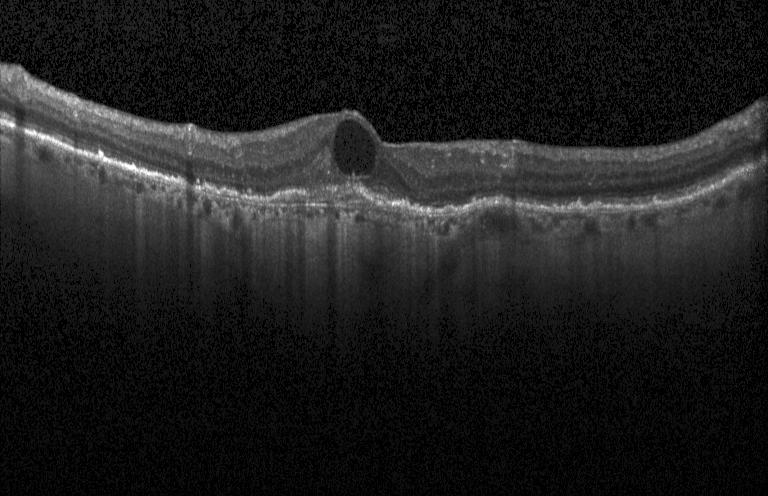

Impression: a choroidal neovascular membrane.